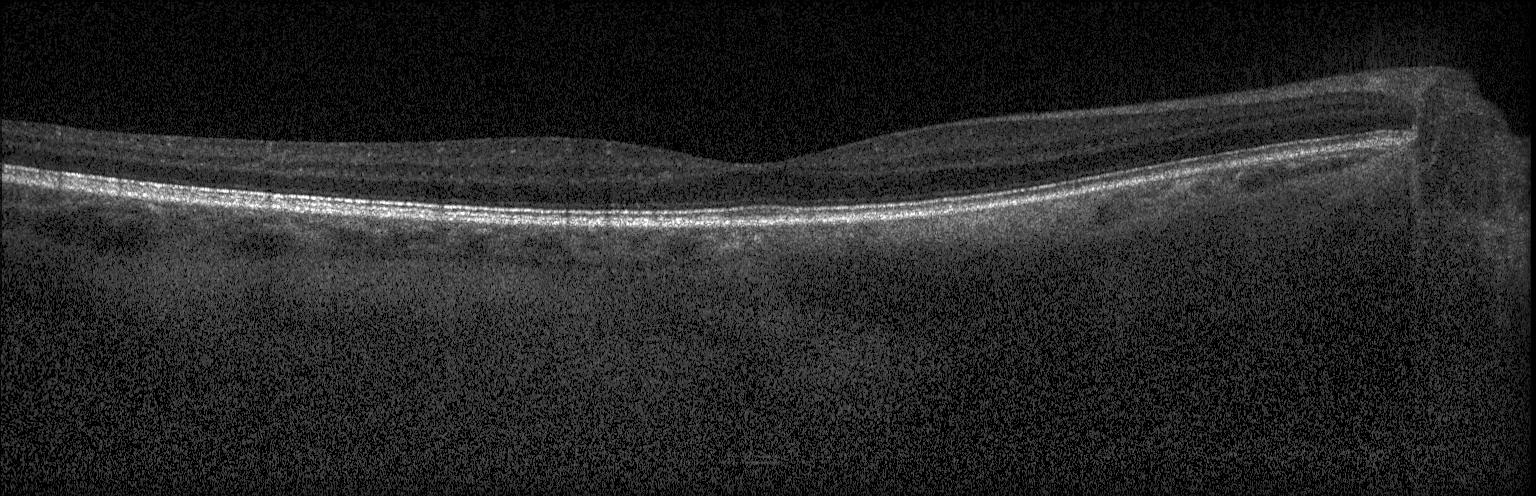
Optical coherence tomography scan
The scan shows no CNV, DME, or drusen.